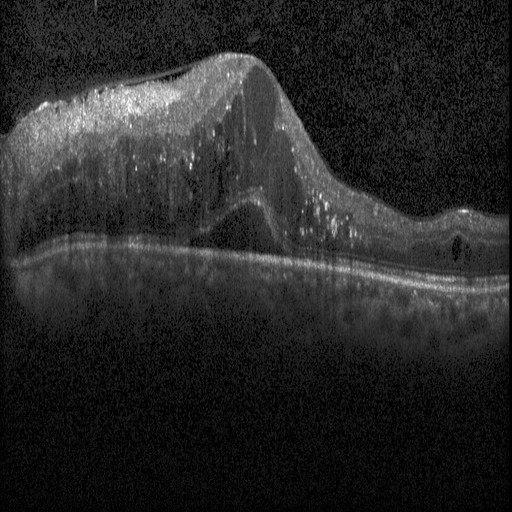
Macular scan · OCT B-scan — This B-scan demonstrates diabetic macular edema (DME).